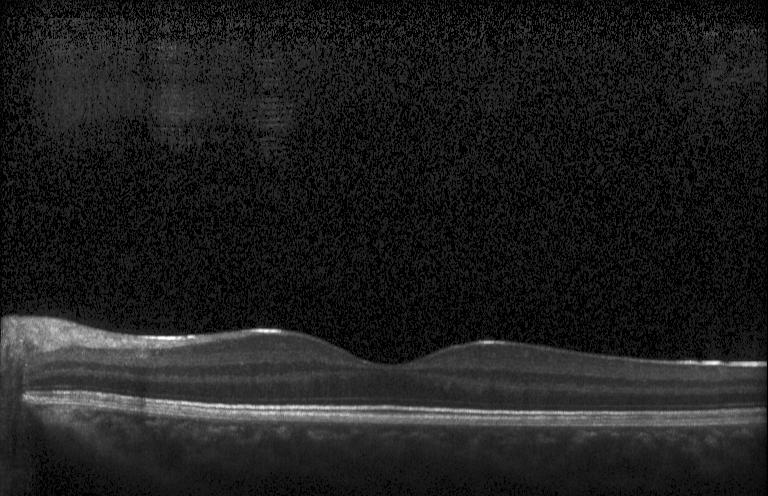 Retinal OCT cross-section. Finding: no choroidal neovascularization, diabetic macular edema, or drusen.